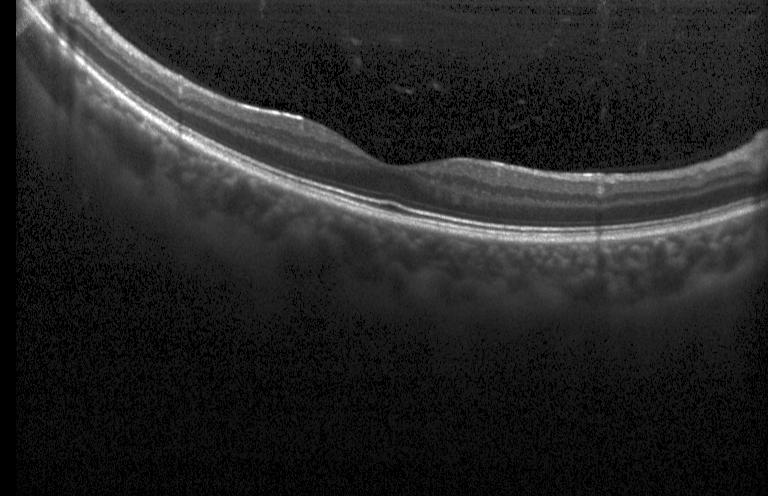 OCT B-scan showing neither CNV, DME, nor drusen.